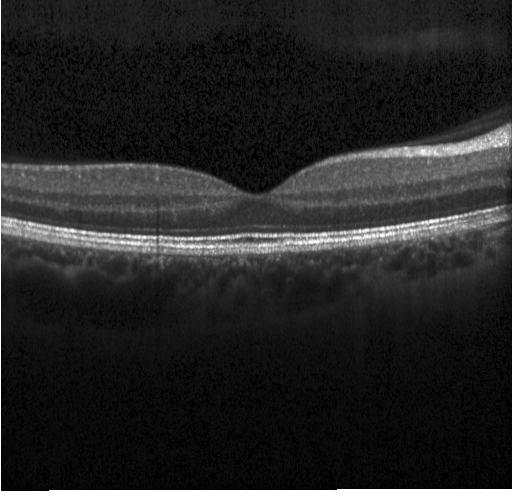 OCT line scan. Impression: no choroidal neovascularization, diabetic macular edema, or drusen.